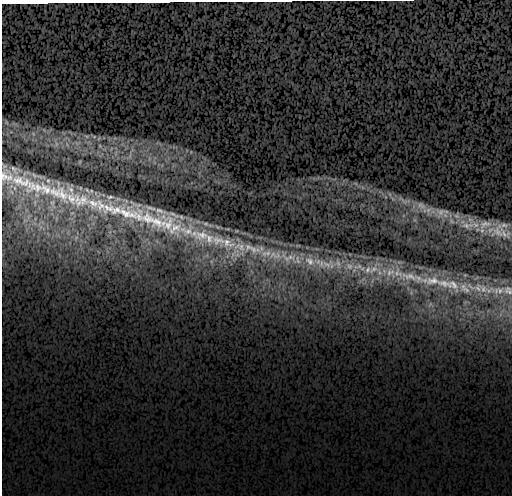
Spectral-domain optical coherence tomography. Retinal OCT B-scan. Centered on the fovea. This B-scan demonstrates no choroidal neovascularization, no diabetic macular edema, and no drusen.